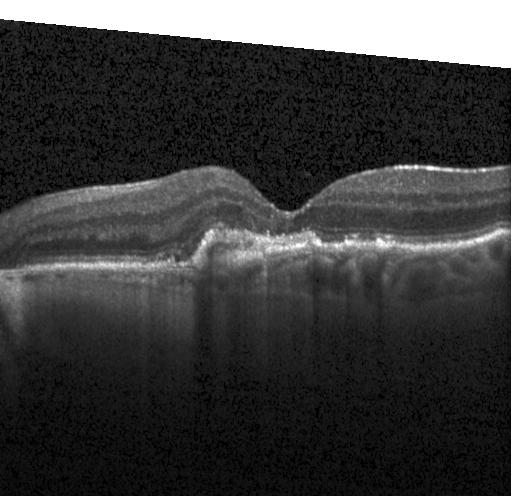 Spectral-domain OCT, optical coherence tomography B-scan
Assessment: choroidal neovascularization (CNV).